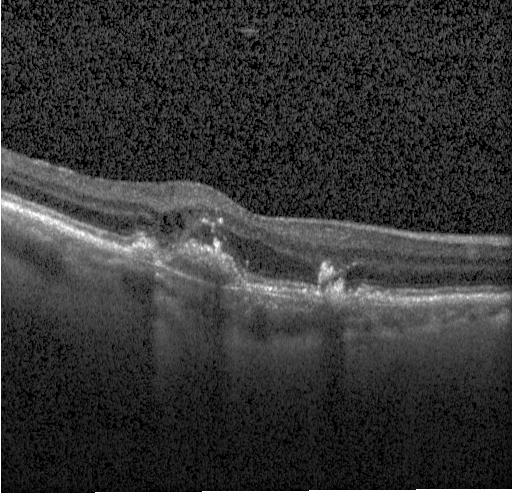
Centered on the fovea; acquired on a Heidelberg Spectralis; retinal OCT cross-section; spectral-domain OCT.
Macular OCT: choroidal neovascularization.